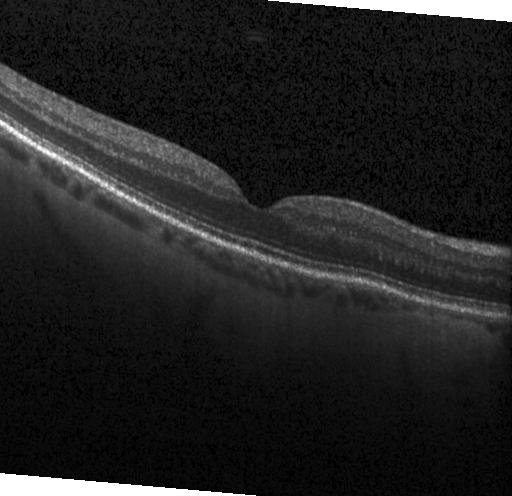

Through the macula, retinal OCT cross-section
This B-scan demonstrates no evidence of choroidal neovascularization, diabetic macular edema, or drusen.